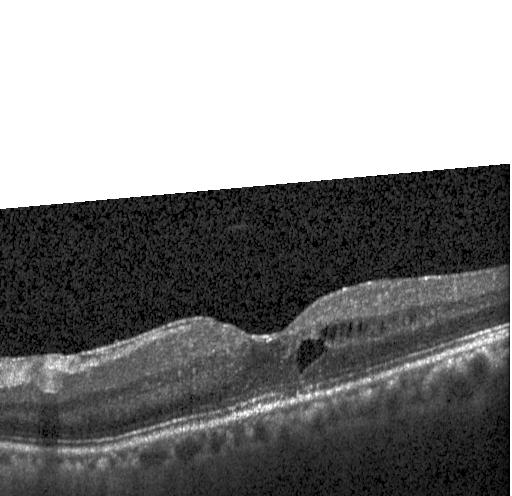

Dx: DME.